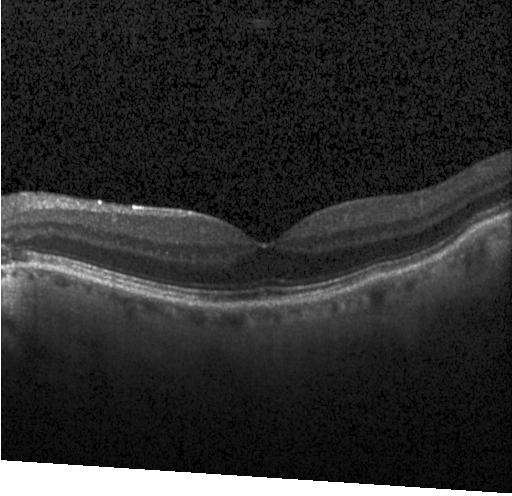
Retinal OCT cross-section · centered on the fovea · acquired on a Heidelberg Spectralis.
Finding: no CNV, DME, or drusen.